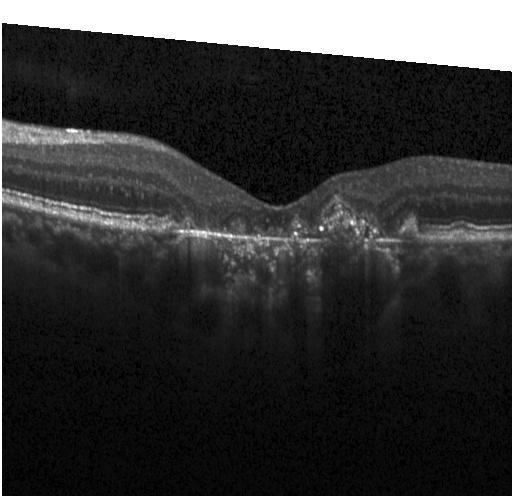

OCT line scan.
Dx: a choroidal neovascular membrane.